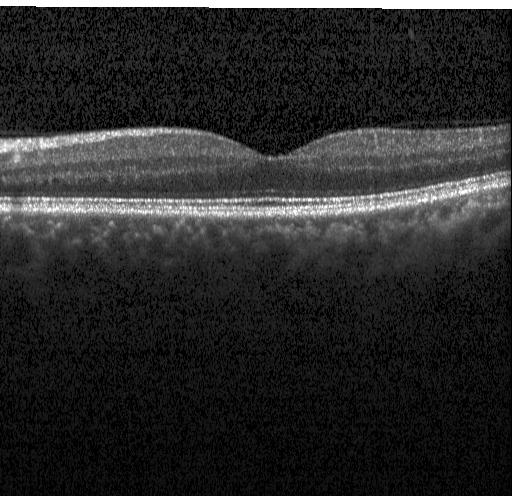

Optical coherence tomography B-scan; through the macula; Heidelberg Spectralis; SD-OCT. Impression: no choroidal neovascularization, no diabetic macular edema, and no drusen.